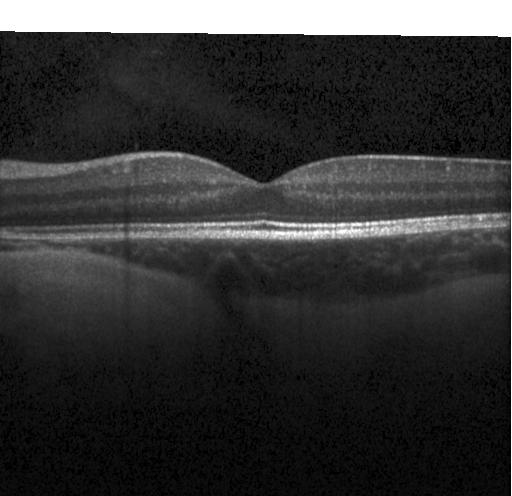 OCT line scan. Through the macula. Spectral-domain optical coherence tomography. Heidelberg Spectralis OCT system.
The scan shows neither choroidal neovascularization, diabetic macular edema, nor drusen.